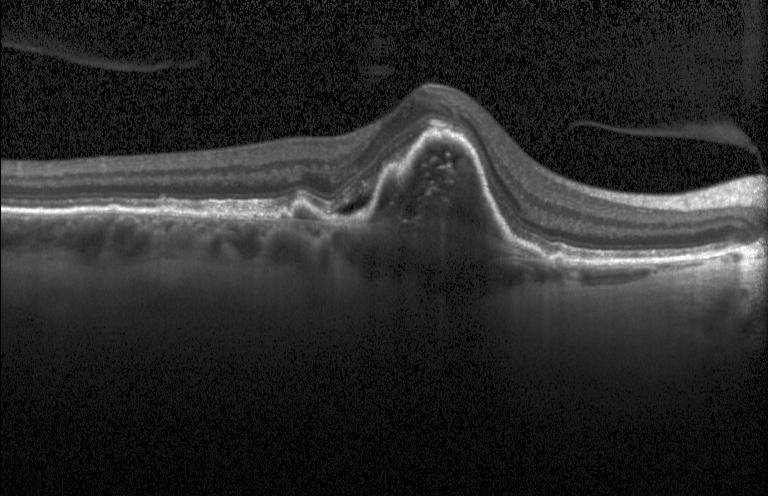
Retinal OCT cross-section
Finding: CNV.